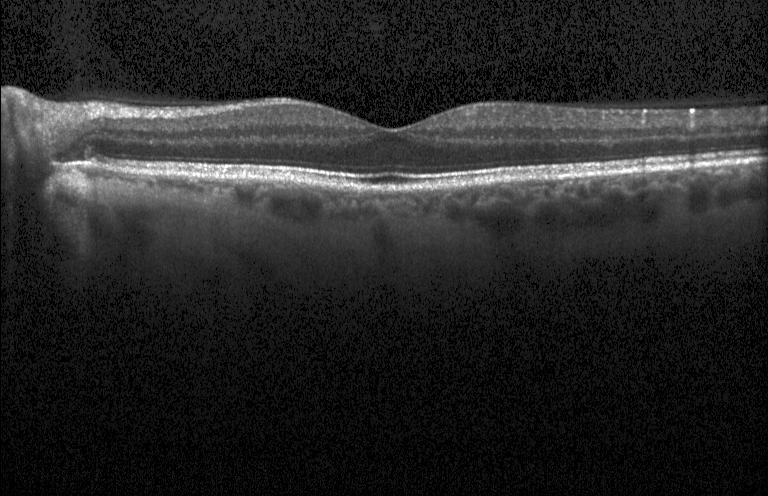

Macular OCT demonstrating neither choroidal neovascularization, diabetic macular edema, nor drusen.